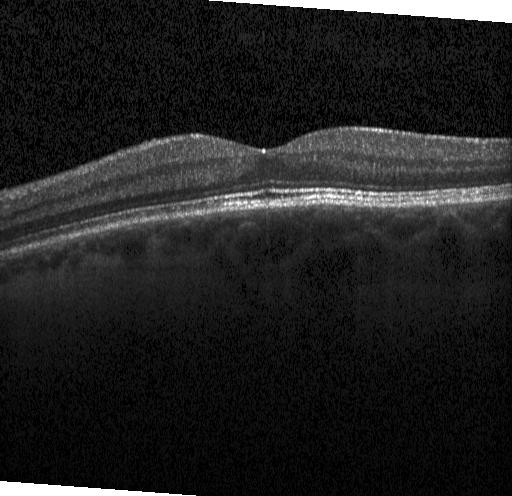

Finding: no evidence of choroidal neovascularization, diabetic macular edema, or drusen.